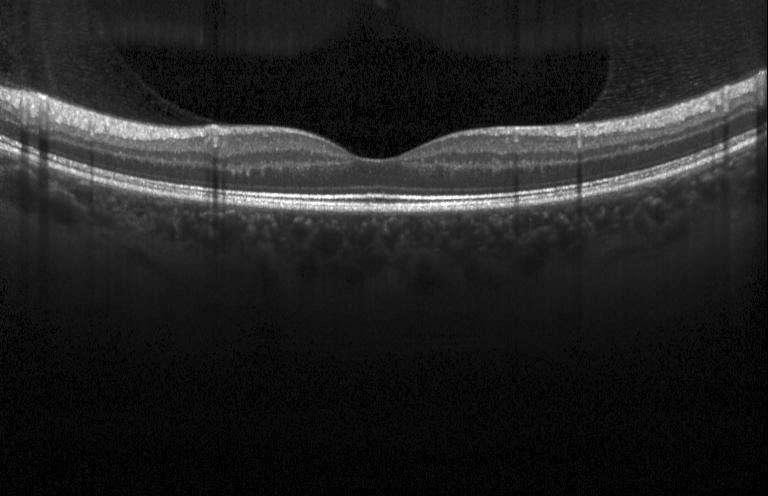
Macular OCT demonstrating neither choroidal neovascularization, diabetic macular edema, nor drusen.